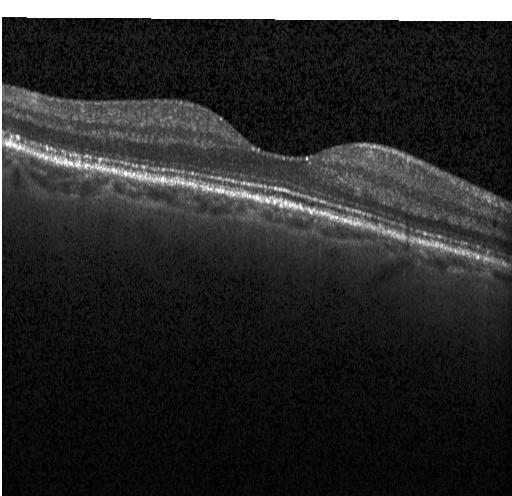 Finding: no evidence of CNV, DME, or drusen.